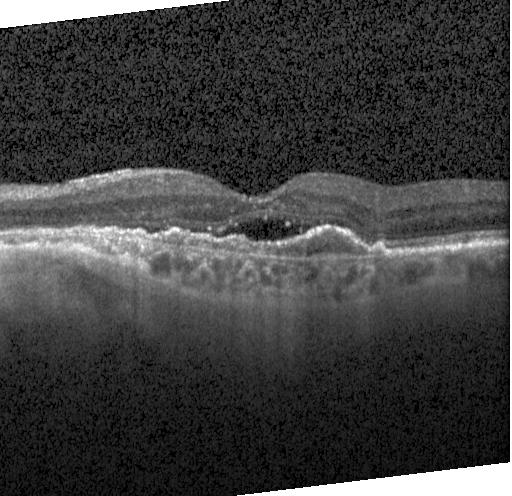
Heidelberg Spectralis. Macular scan. Spectral-domain optical coherence tomography. Retinal OCT cross-section
Assessment: a choroidal neovascular membrane.